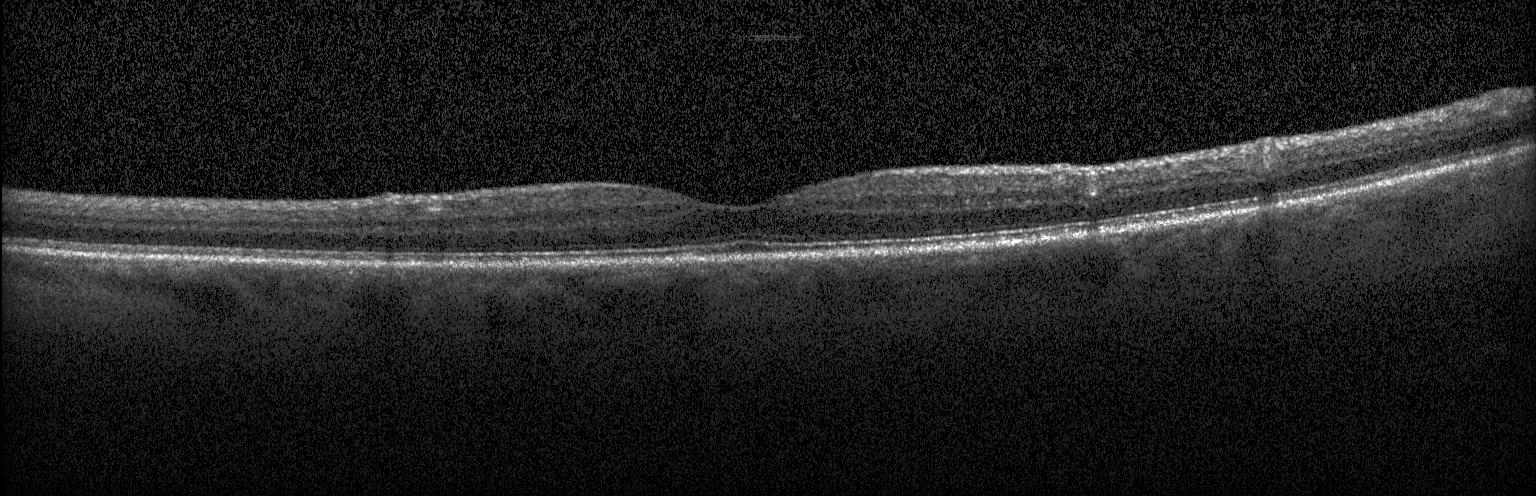

Assessment: no choroidal neovascularization, no diabetic macular edema, and no drusen.